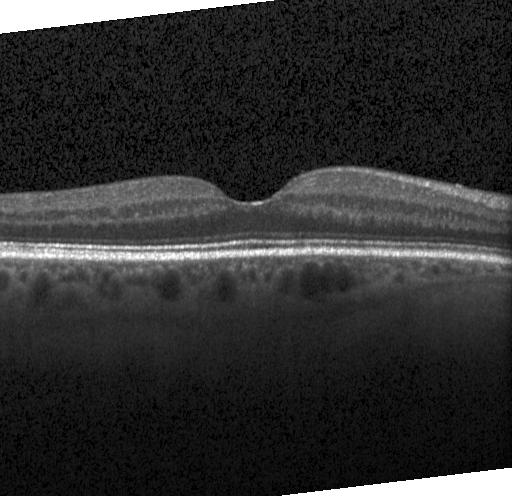

Fovea-centered · spectral-domain OCT · acquired on a Heidelberg Spectralis · optical coherence tomography scan.
OCT finding: neither choroidal neovascularization, diabetic macular edema, nor drusen.